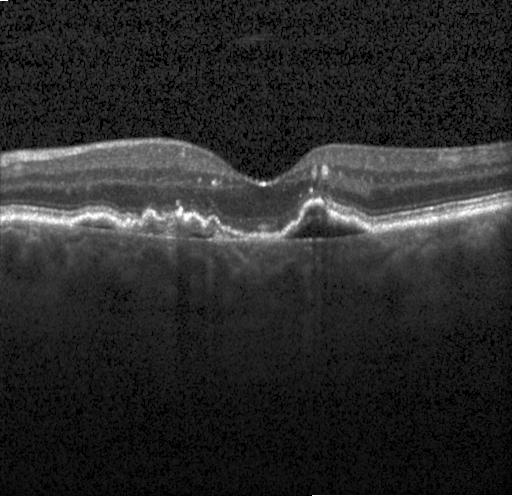
Assessment: CNV.